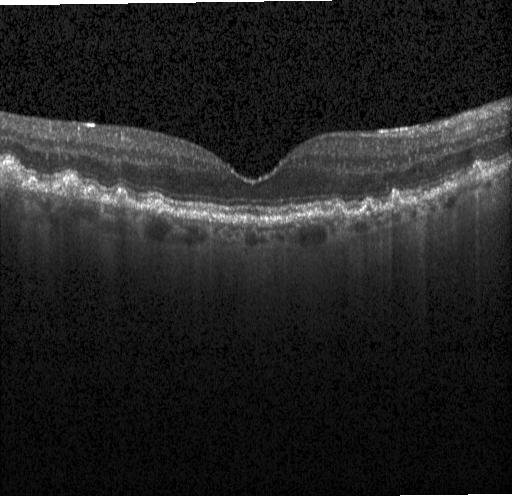 Finding: multiple drusen.